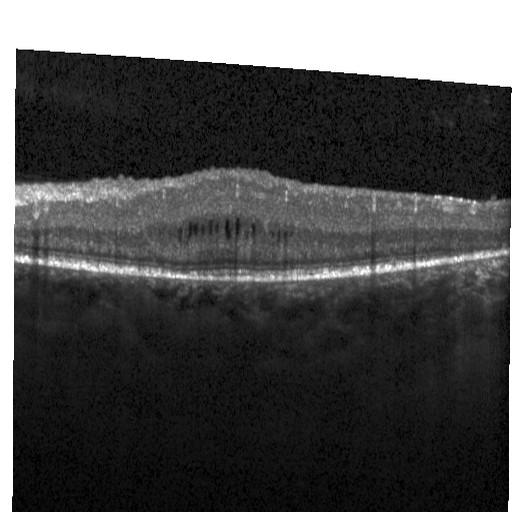

Optical coherence tomography scan · instrument: Heidelberg Spectralis — Assessment: diabetic macular edema (DME).